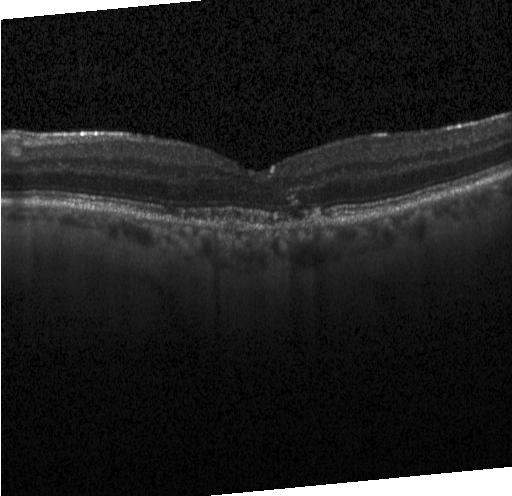
Optical coherence tomography scan
Diagnosis: a choroidal neovascular membrane.